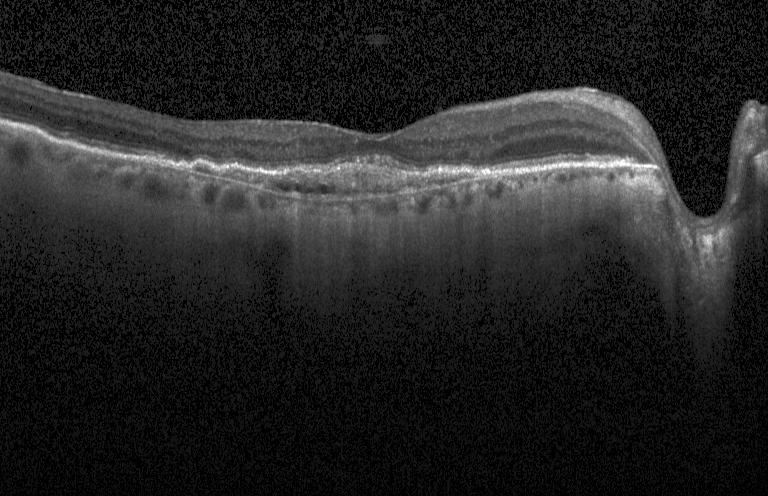

Dx: choroidal neovascularization (CNV).